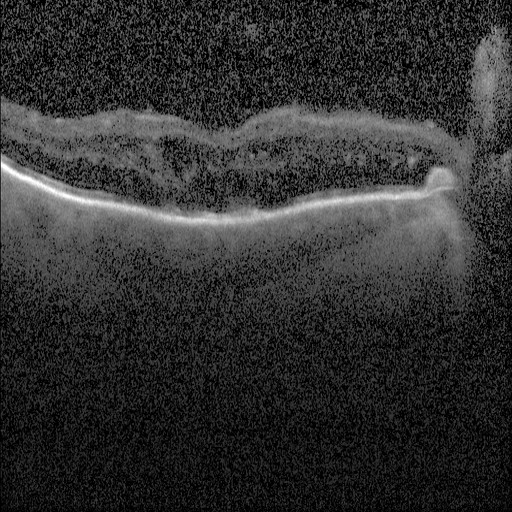

Heidelberg Spectralis OCT system · SD-OCT · optical coherence tomography B-scan · through the macula. This B-scan demonstrates DME.